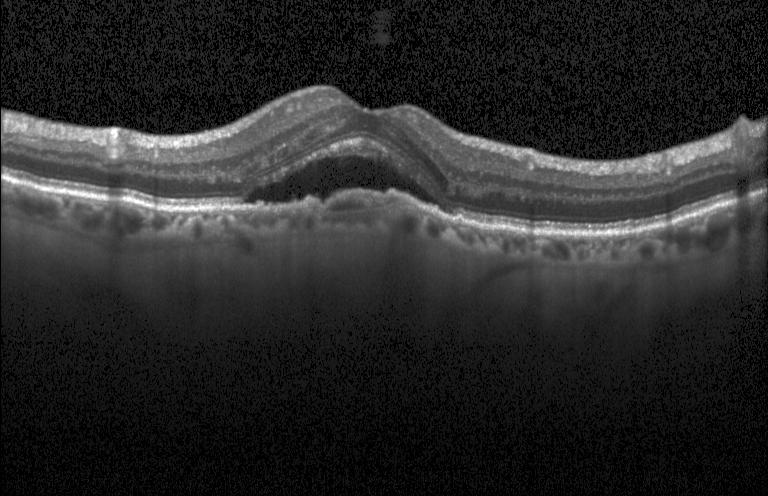
Fovea-centered, SD-OCT, retinal OCT B-scan
The scan shows CNV.